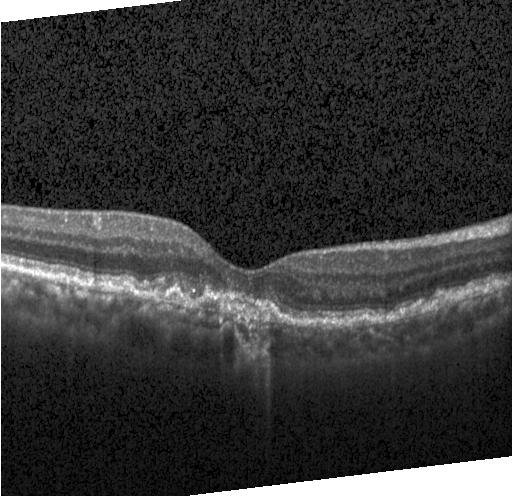
Spectral-domain OCT. Macular scan. Retinal OCT B-scan. Acquired on a Heidelberg Spectralis. The scan shows choroidal neovascularization.